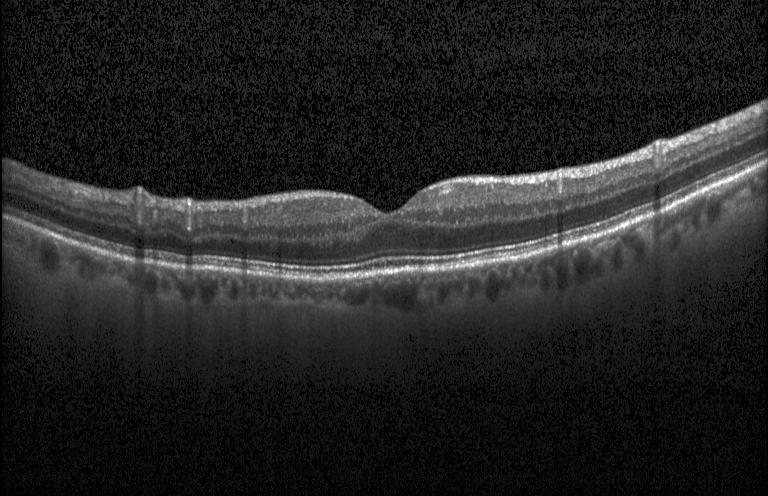

SD-OCT. Optical coherence tomography scan.
This B-scan demonstrates no choroidal neovascularization, diabetic macular edema, or drusen.